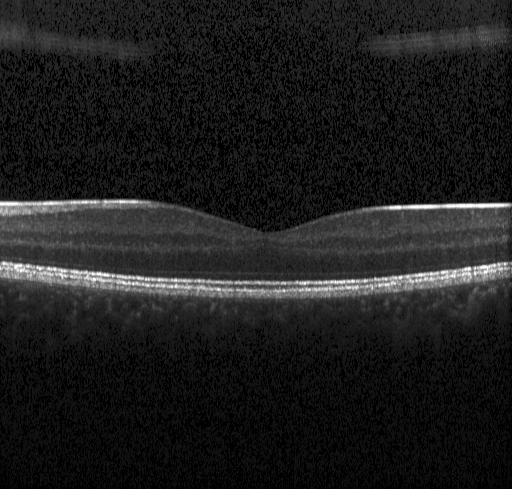 Assessment: no choroidal neovascularization, diabetic macular edema, or drusen.